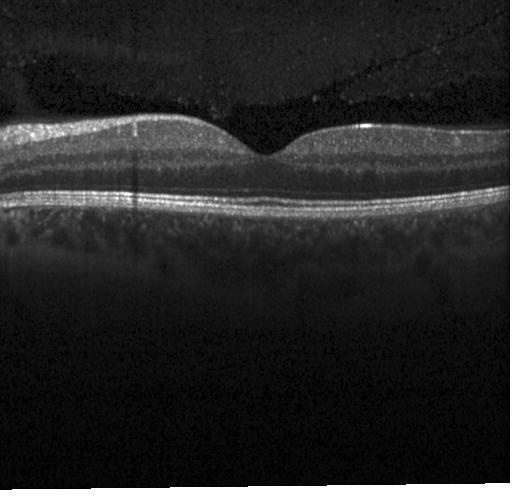 OCT finding: no CNV, DME, or drusen.